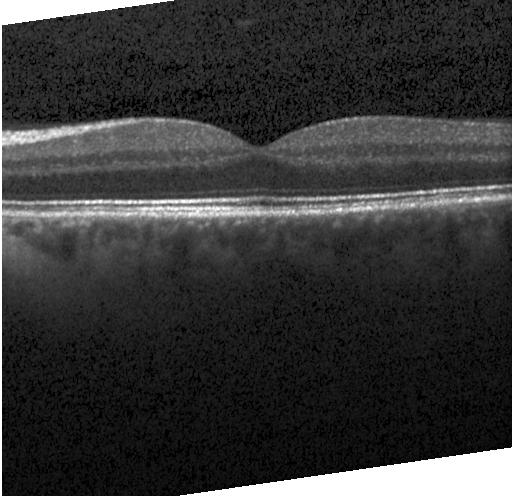

Diagnosis: neither CNV, DME, nor drusen.